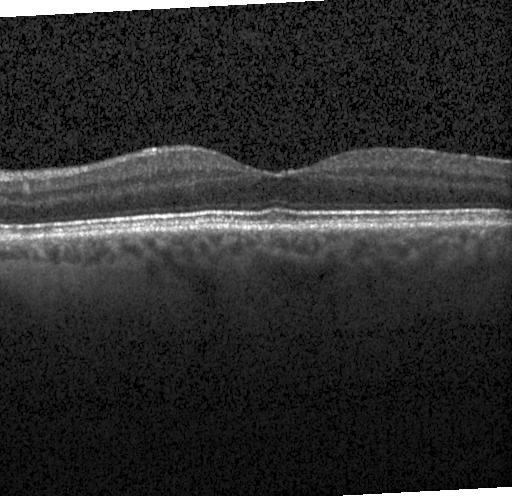

Spectral-domain optical coherence tomography, horizontal scan through the fovea, OCT line scan, instrument: Heidelberg Spectralis — Finding: neither choroidal neovascularization, diabetic macular edema, nor drusen.